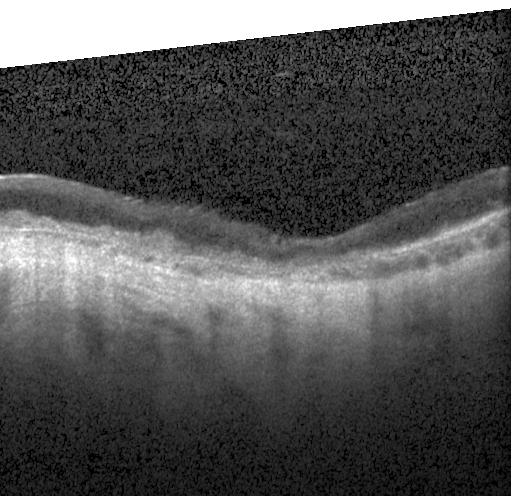 Macular OCT demonstrating CNV.